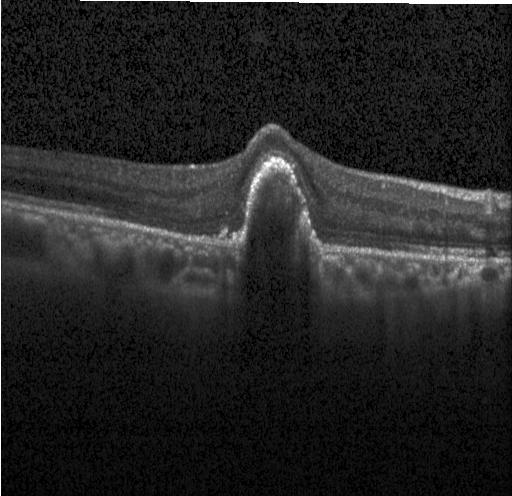

Retinal OCT cross-section showing a choroidal neovascular membrane.